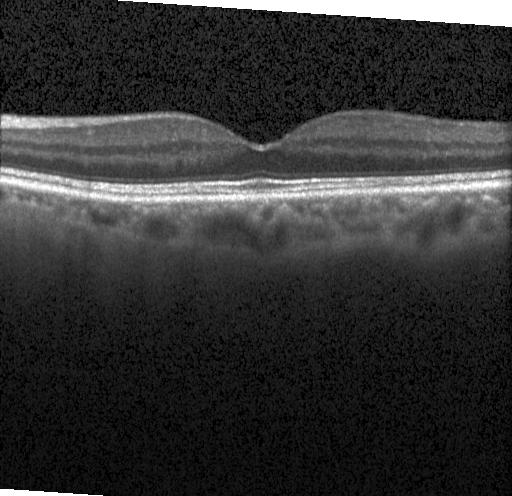 Heidelberg Spectralis; retinal OCT B-scan; fovea-centered.
No choroidal neovascularization, diabetic macular edema, or drusen.